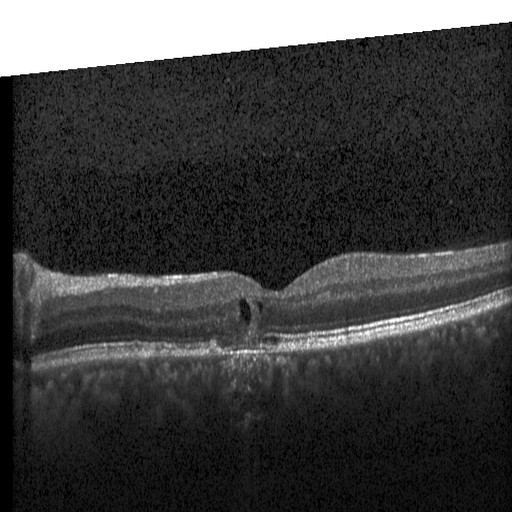
Centered on the fovea, spectral-domain OCT, retinal OCT cross-section.
DME.